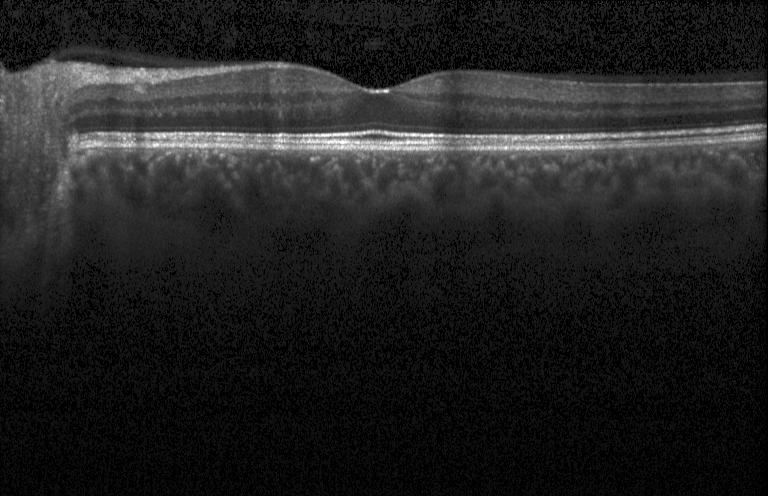
OCT line scan · Heidelberg Spectralis · centered on the fovea.
OCT finding: no CNV, no DME, and no drusen.